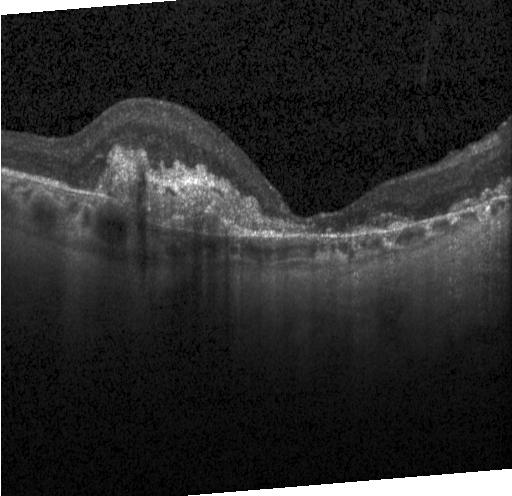 The scan shows a choroidal neovascular membrane.